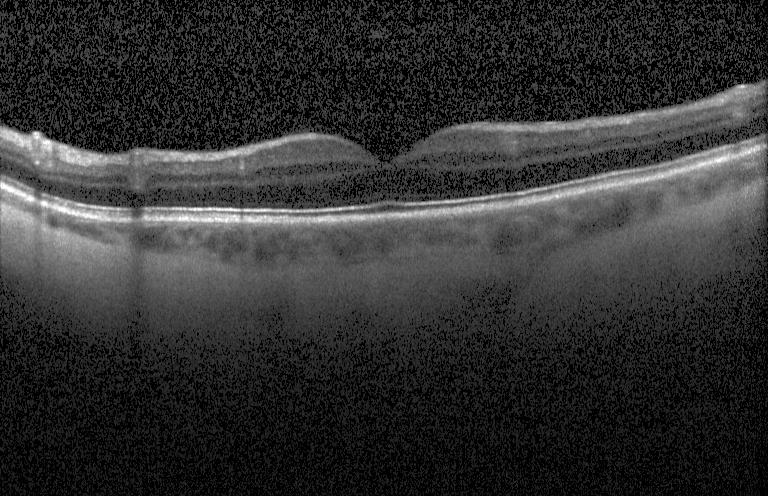 Retinal OCT cross-section. SD-OCT. Heidelberg Spectralis OCT system. Fovea-centered
This B-scan demonstrates neither choroidal neovascularization, diabetic macular edema, nor drusen.